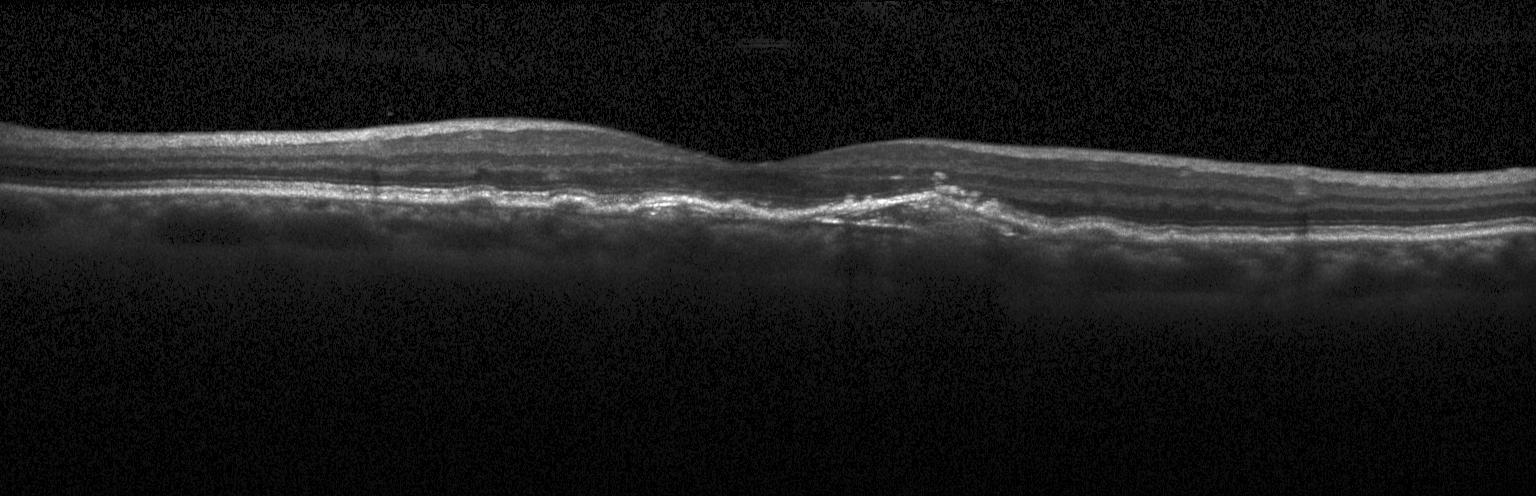

Spectral-domain OCT · optical coherence tomography B-scan — Diagnosis: a choroidal neovascular membrane.